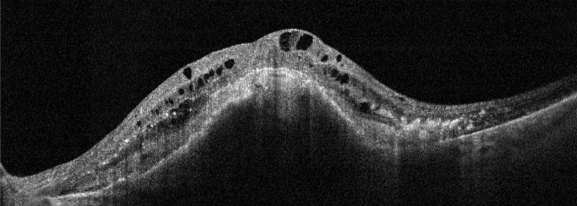

Spectral-domain OCT B-scan: age-related macular degeneration.